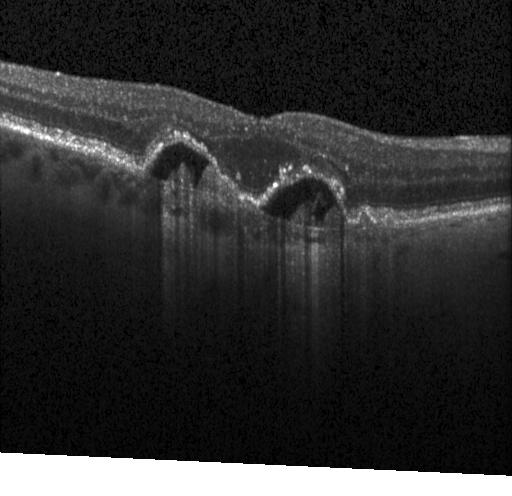
Through the macula, optical coherence tomography scan, acquired on a Heidelberg Spectralis — Dx: a choroidal neovascular membrane.